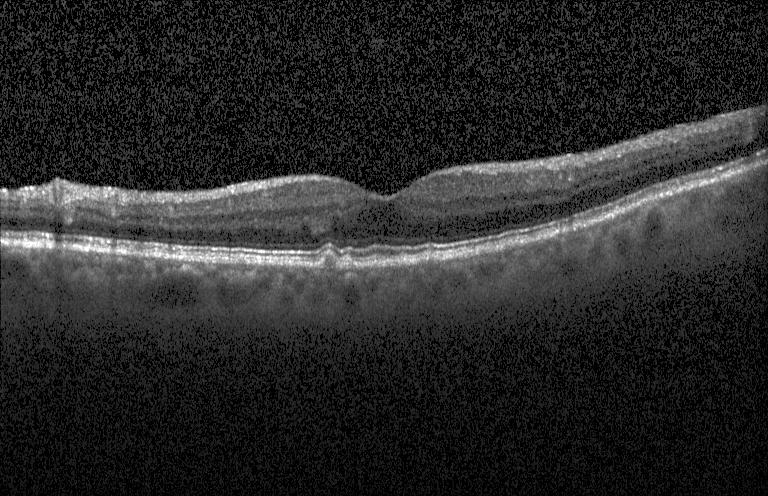

Retinal OCT B-scan · instrument: Heidelberg Spectralis. Sub-RPE drusenoid deposits.